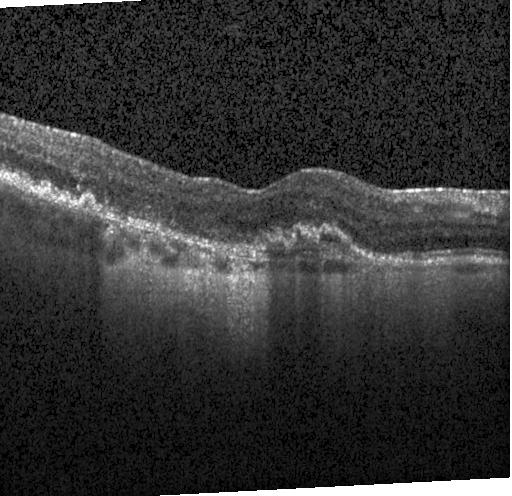 SD-OCT. OCT B-scan.
Impression: a choroidal neovascular membrane.